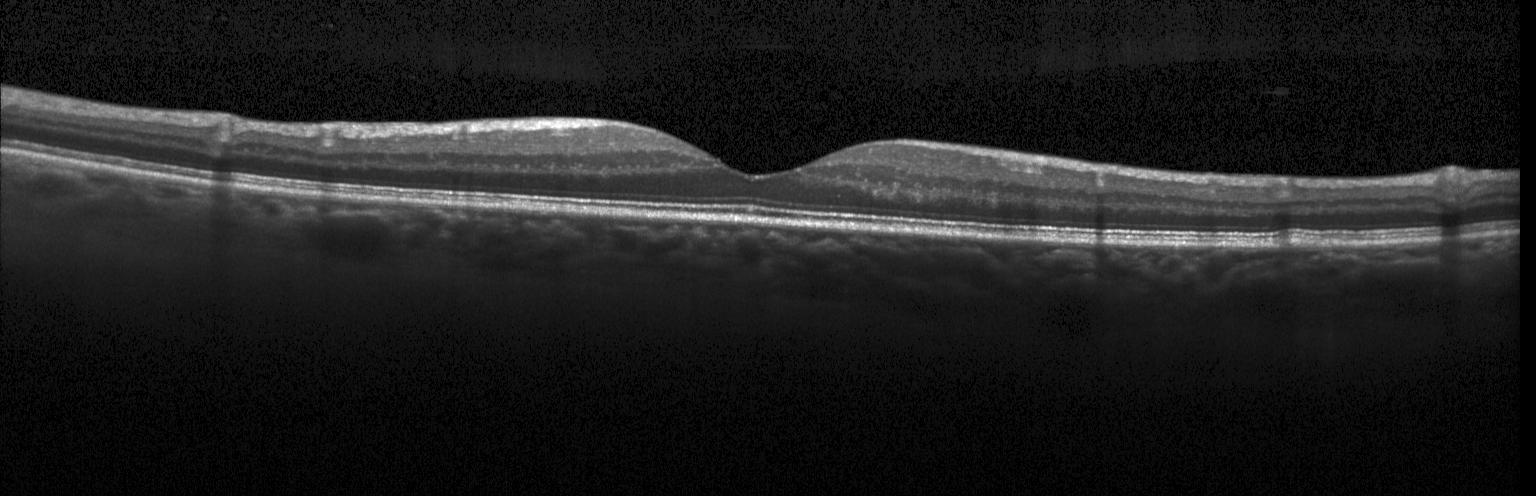
Optical coherence tomography scan — Assessment: no choroidal neovascularization, diabetic macular edema, or drusen.